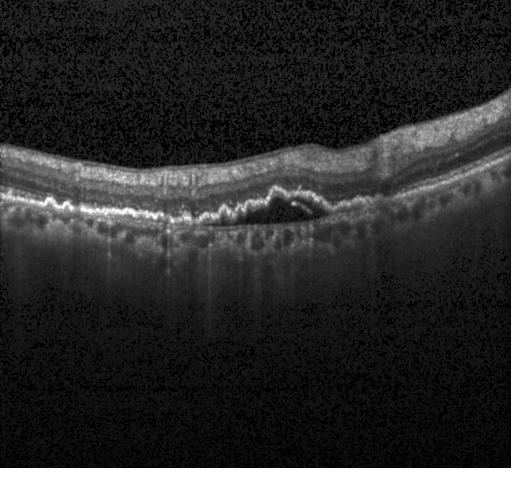
OCT line scan
Finding: choroidal neovascularization.